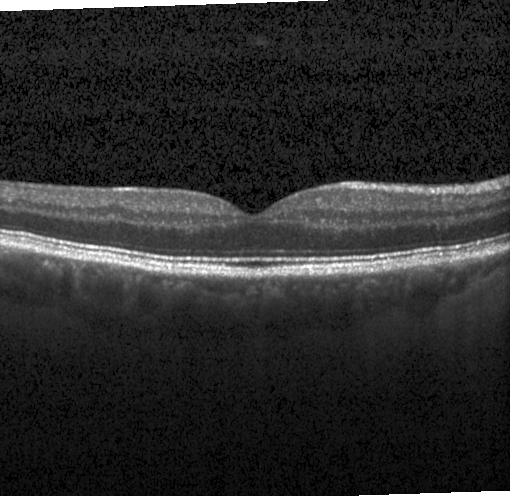
Retinal OCT cross-section — The scan shows no choroidal neovascularization, no diabetic macular edema, and no drusen.